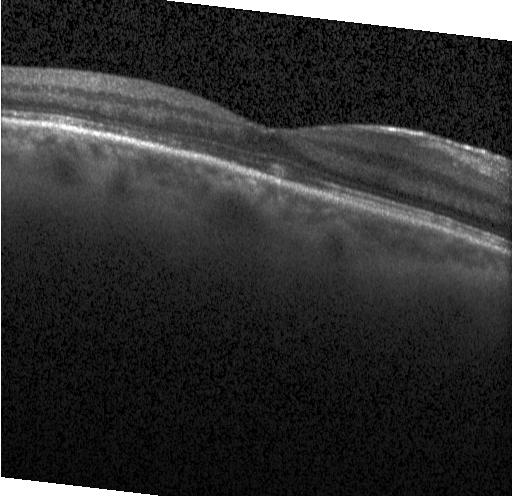
Heidelberg Spectralis. Centered on the fovea. Optical coherence tomography B-scan.
Diagnosis: no evidence of CNV, DME, or drusen.